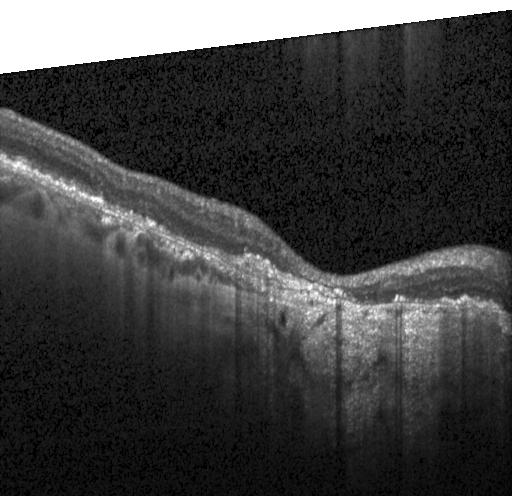
Acquired on a Heidelberg Spectralis; retinal OCT cross-section. Diagnosis: a choroidal neovascular membrane.